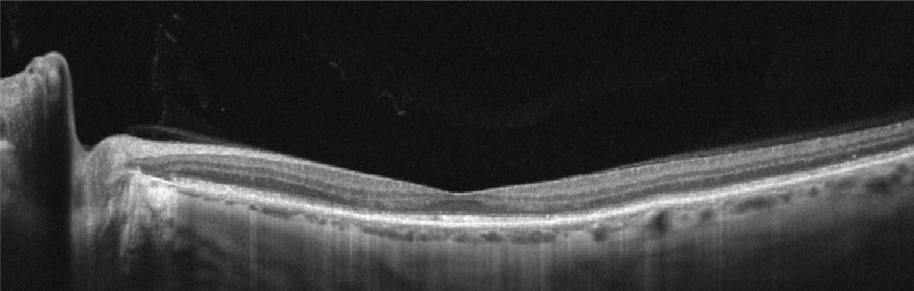 Acquired on an Optovue Avanti RTVue XR, optical coherence tomography scan. Finding: age-related macular degeneration.